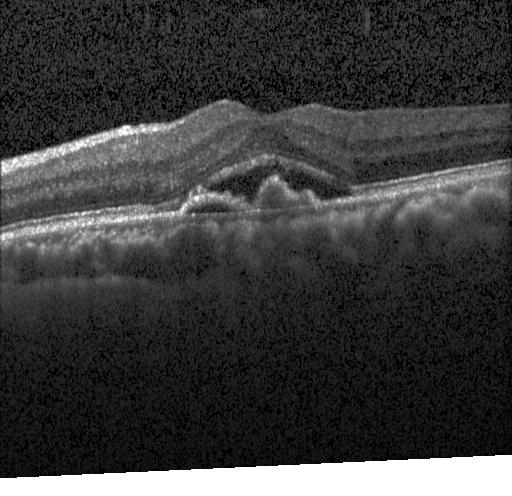 Macular OCT demonstrating choroidal neovascularization.